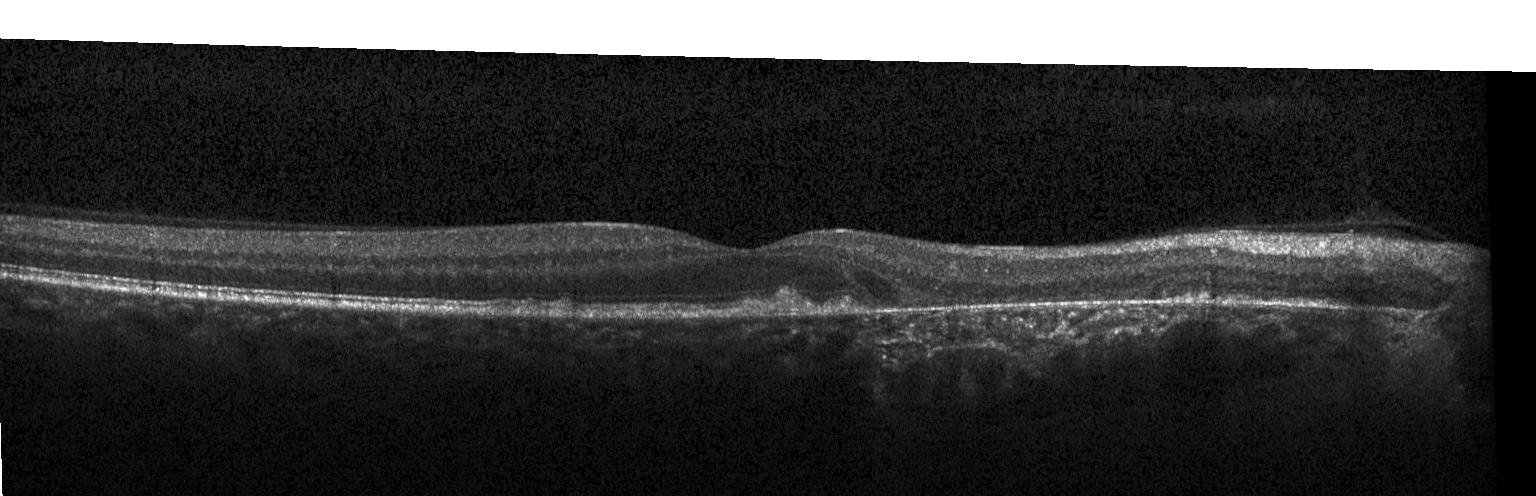
Acquired on a Heidelberg Spectralis. Horizontal scan through the fovea. OCT B-scan — Assessment: choroidal neovascularization (CNV).